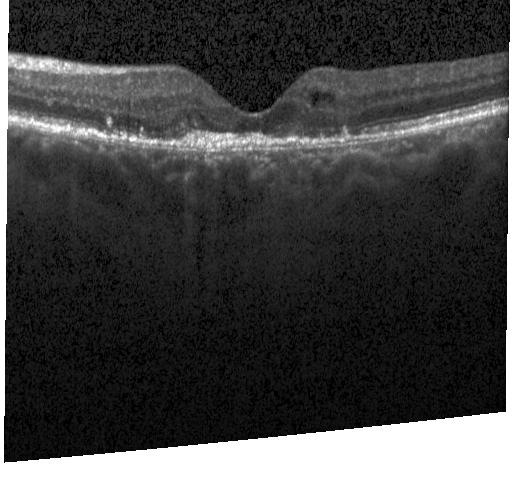

Retinal OCT cross-section showing CNV.